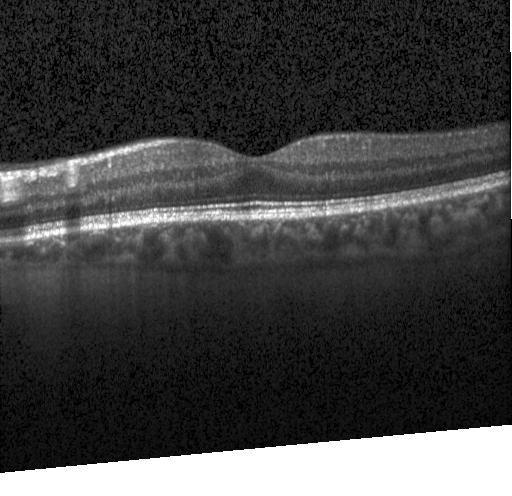 OCT B-scan showing no CNV, no DME, and no drusen.